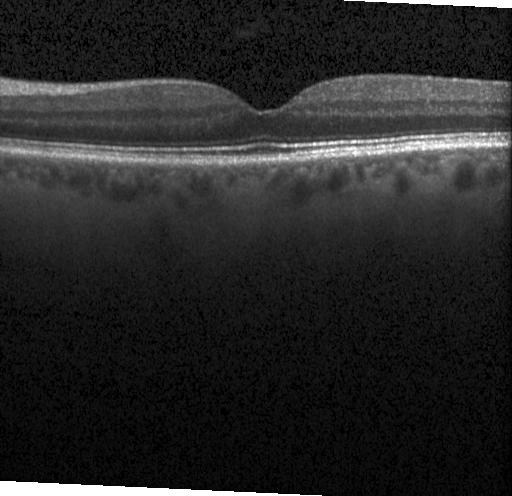 Finding: neither choroidal neovascularization, diabetic macular edema, nor drusen.